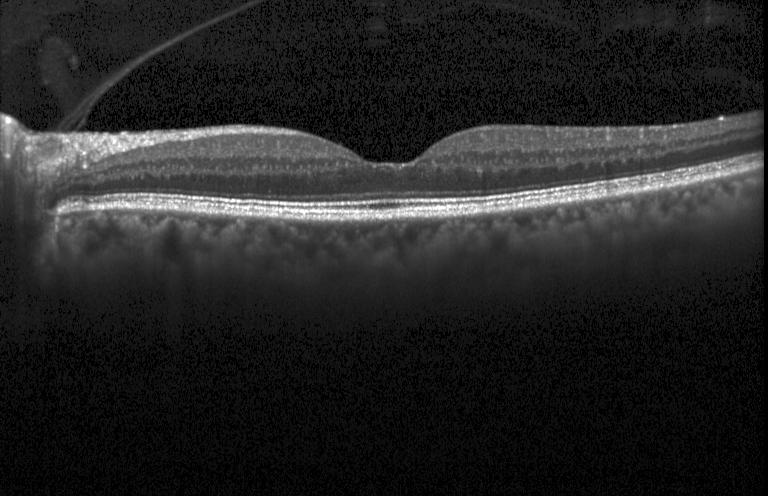 The scan shows neither CNV, DME, nor drusen.